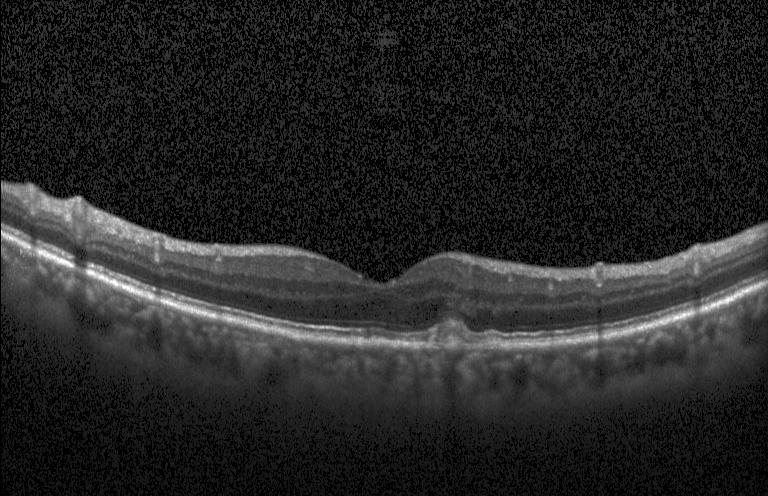
Heidelberg Spectralis OCT system · macular scan · optical coherence tomography B-scan · SD-OCT. Diagnosis: sub-RPE drusenoid deposits.